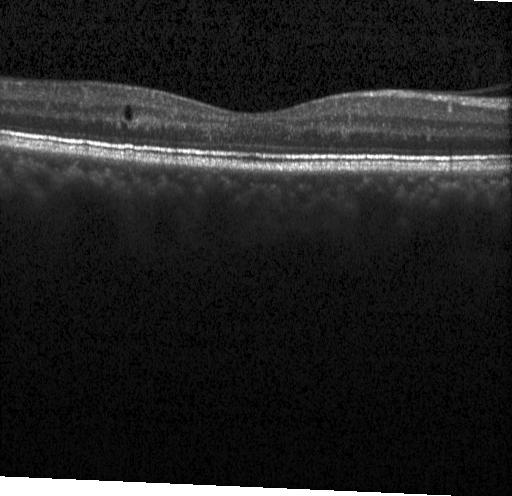 Finding: diabetic macular edema.